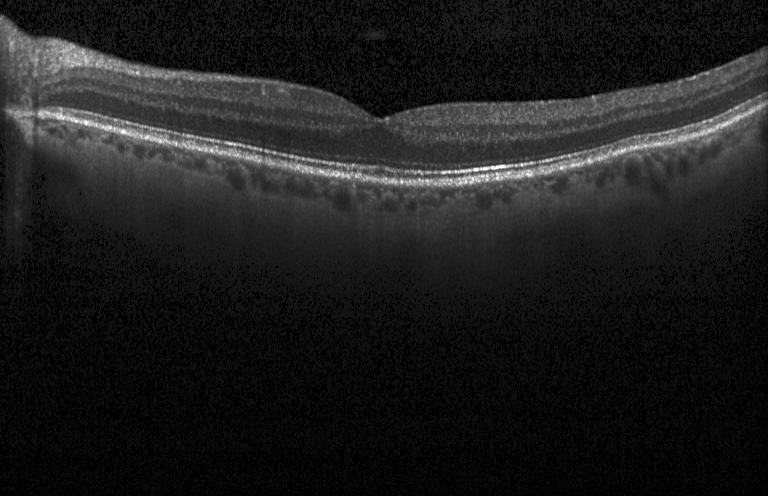

SD-OCT; fovea-centered; retinal OCT cross-section; acquired on a Heidelberg Spectralis
Diagnosis: no evidence of CNV, DME, or drusen.